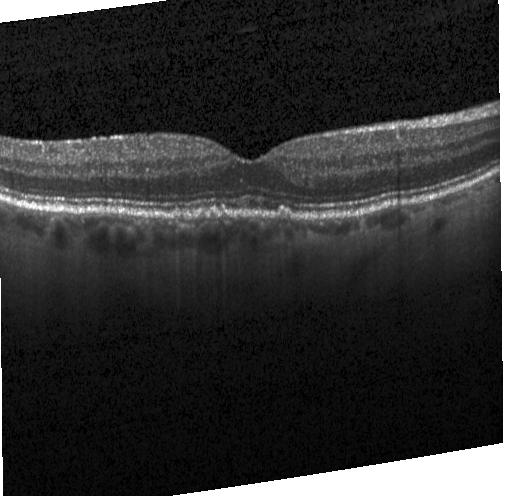
This B-scan demonstrates drusen.